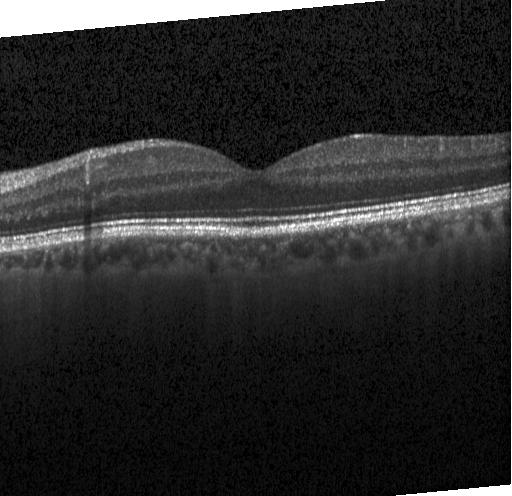

Instrument: Heidelberg Spectralis, OCT line scan
Impression: no CNV, DME, or drusen.